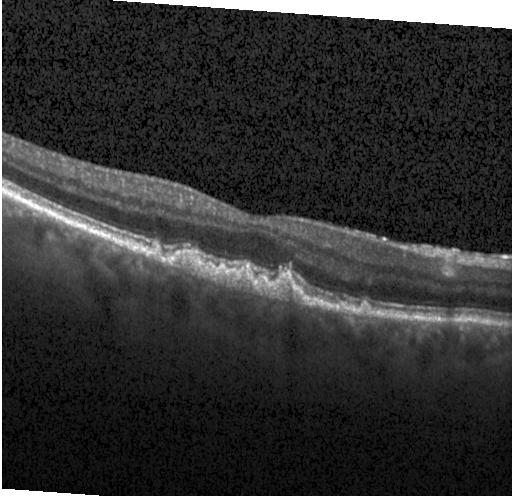

OCT B-scan. SD-OCT. Macular scan. This B-scan demonstrates sub-RPE drusenoid deposits.